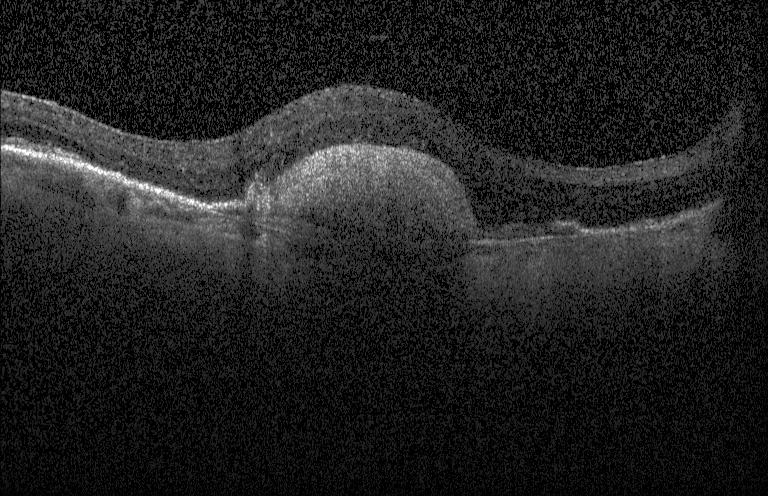
Optical coherence tomography B-scan — Assessment: a choroidal neovascular membrane.